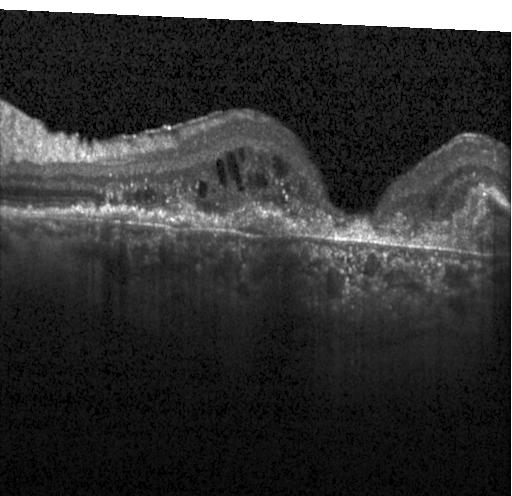

OCT line scan, spectral-domain OCT. Impression: choroidal neovascularization (CNV).